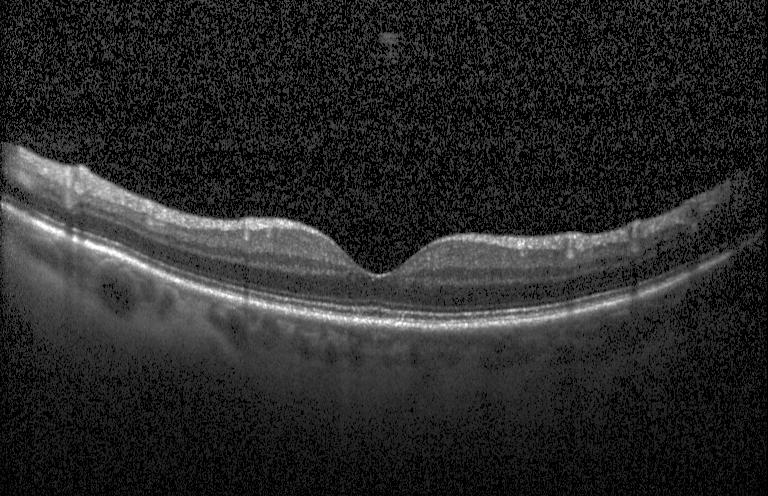
Optical coherence tomography B-scan. Impression: neither choroidal neovascularization, diabetic macular edema, nor drusen.